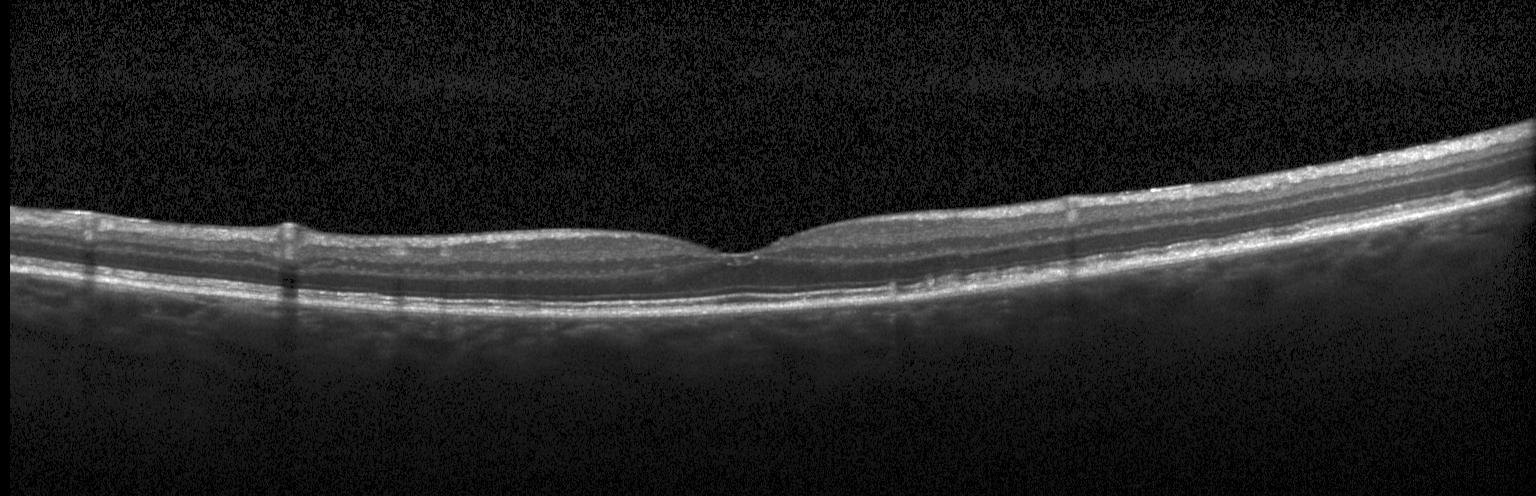

Centered on the fovea; spectral-domain optical coherence tomography; OCT line scan
Impression: multiple drusen.